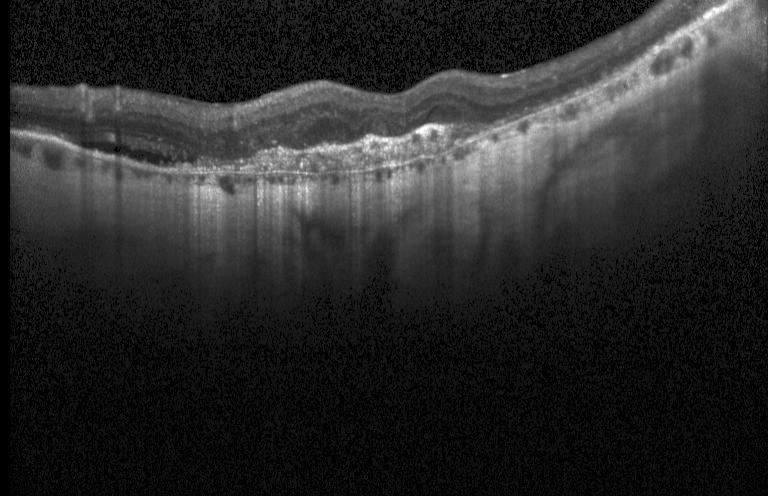

Choroidal neovascularization.